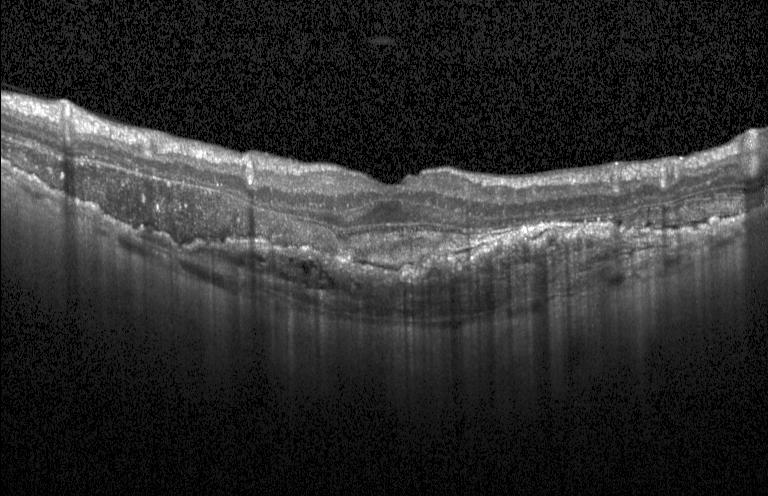 Diagnosis: a choroidal neovascular membrane.